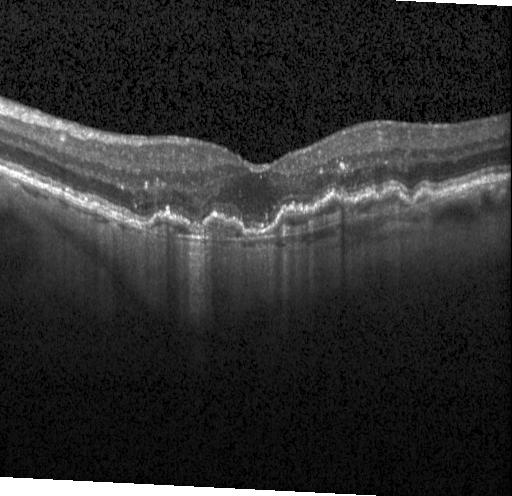

Retinal OCT cross-section.
Dx: a choroidal neovascular membrane.